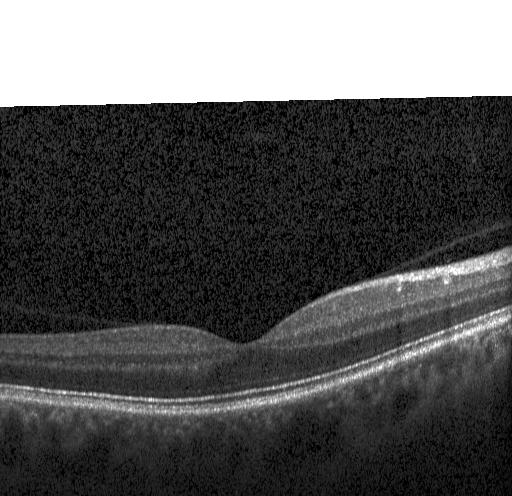 Retinal OCT cross-section — Assessment: no evidence of choroidal neovascularization, diabetic macular edema, or drusen.